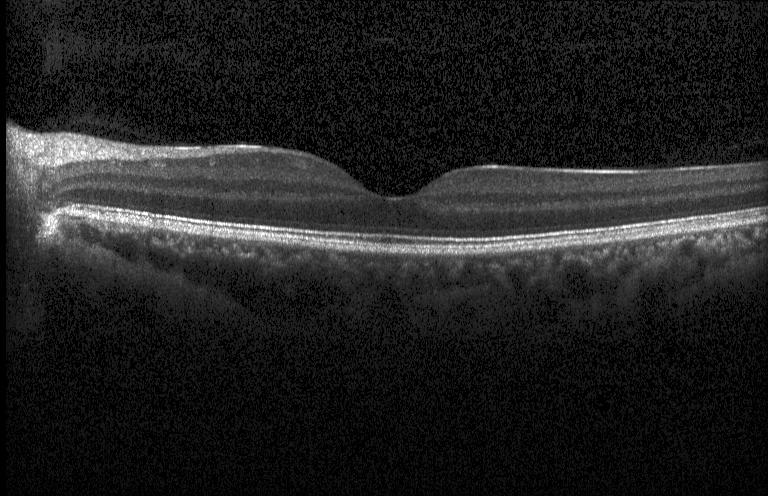

Impression: no choroidal neovascularization, diabetic macular edema, or drusen.